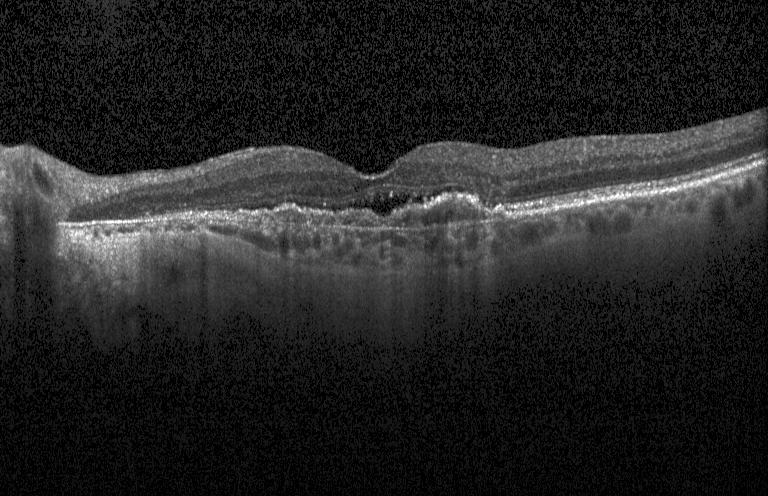
Dx: CNV.